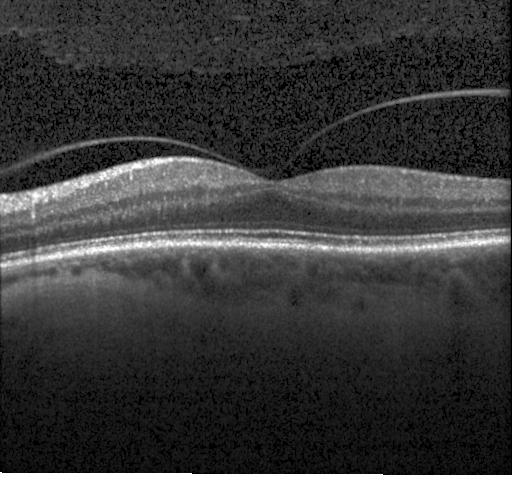

SD-OCT, Heidelberg Spectralis OCT system, macular scan, optical coherence tomography B-scan.
The scan shows no choroidal neovascularization, diabetic macular edema, or drusen.